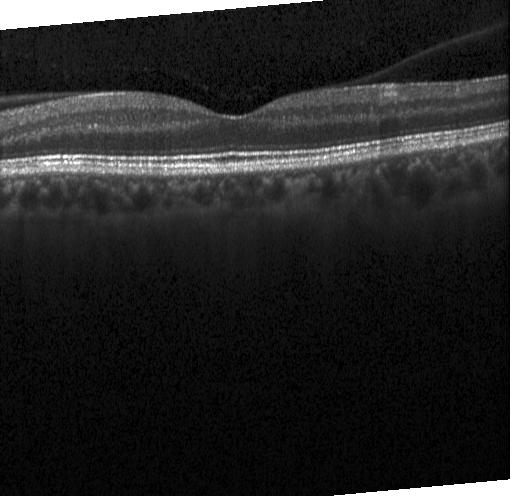
Impression: no evidence of CNV, DME, or drusen.